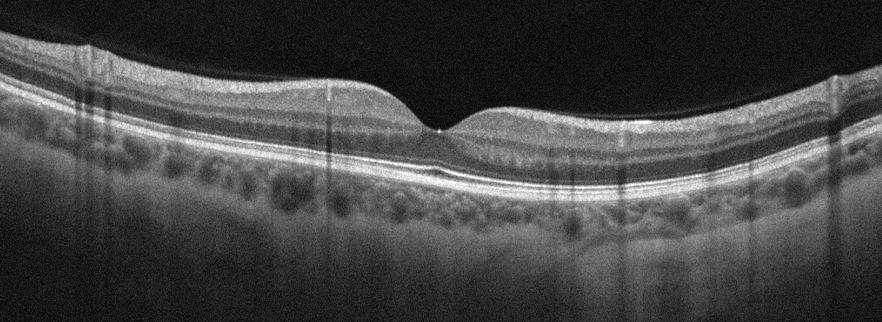

Acquired on an Optovue Avanti RTVue XR, oculus sinister, OCT line scan — No AMD, DME, ERM, RAO, RVO, or VID.